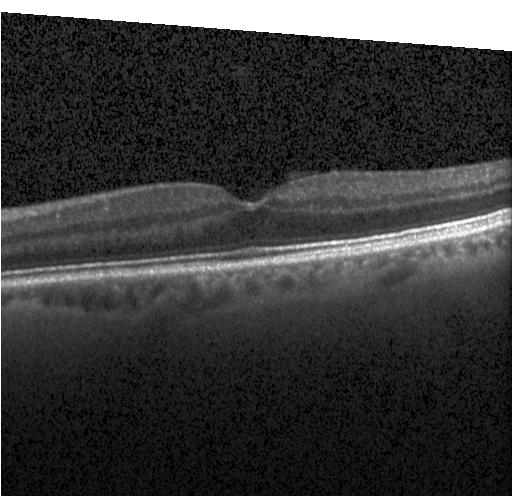

Horizontal scan through the fovea, SD-OCT, instrument: Heidelberg Spectralis, retinal OCT B-scan. Impression: no evidence of choroidal neovascularization, diabetic macular edema, or drusen.